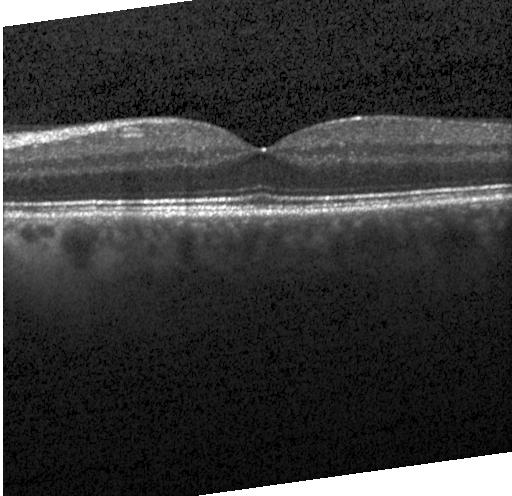

OCT B-scan — Finding: no evidence of CNV, DME, or drusen.